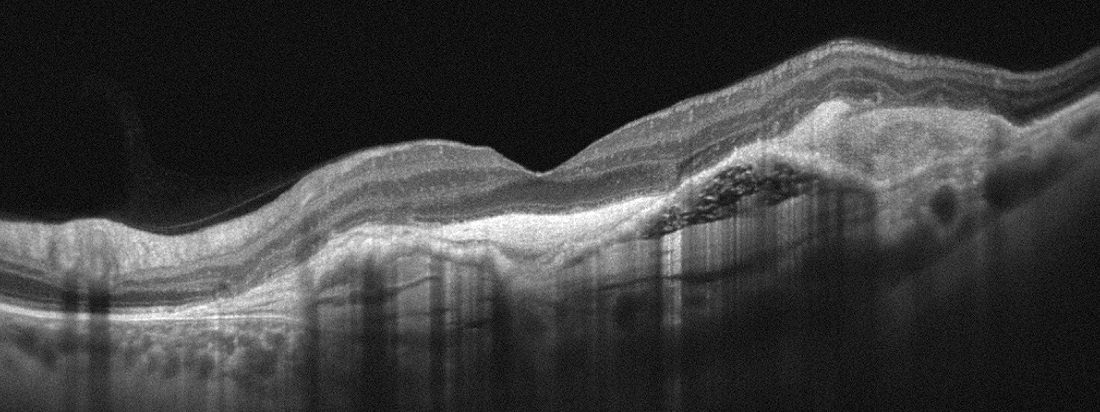

Impression: AMD.